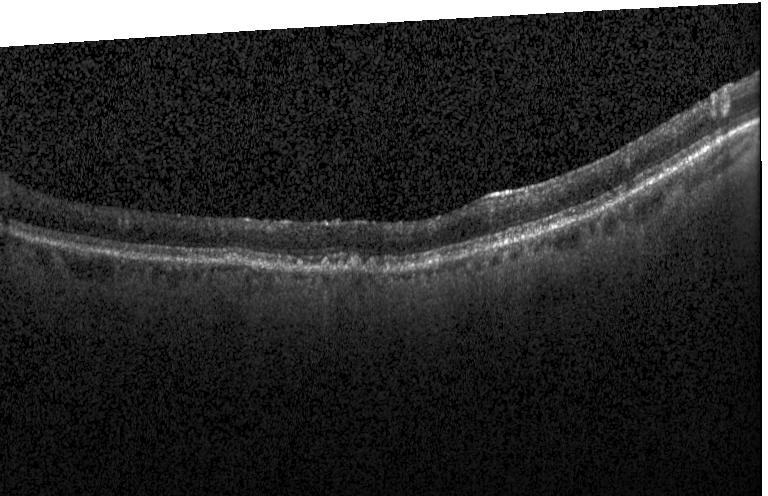
OCT line scan · through the macula. This B-scan demonstrates drusen.